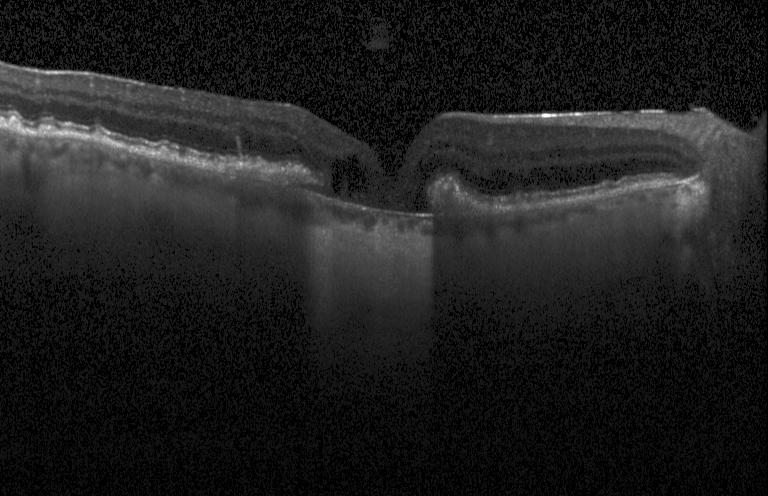

Retinal OCT cross-section. Instrument: Heidelberg Spectralis. Macular scan. SD-OCT — Diagnosis: choroidal neovascularization (CNV).